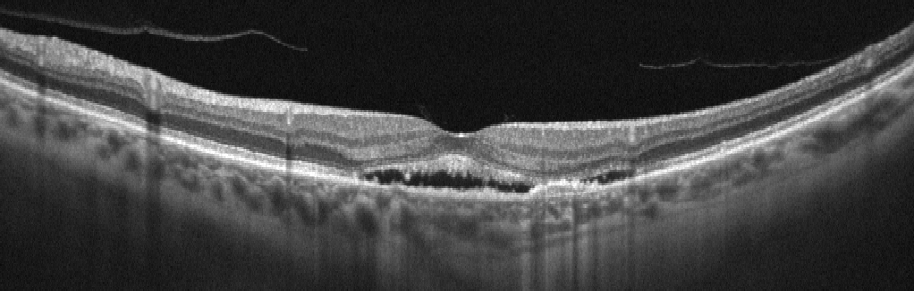 Instrument: Optovue Avanti RTVue XR · optical coherence tomography scan · oculus sinister. Impression: AMD.